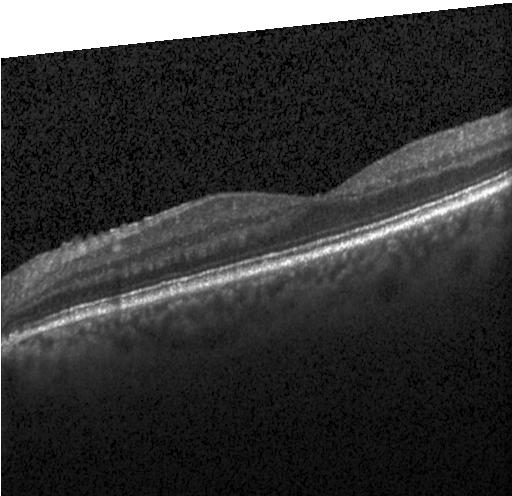 Optical coherence tomography B-scan · centered on the fovea. Assessment: no choroidal neovascularization, no diabetic macular edema, and no drusen.